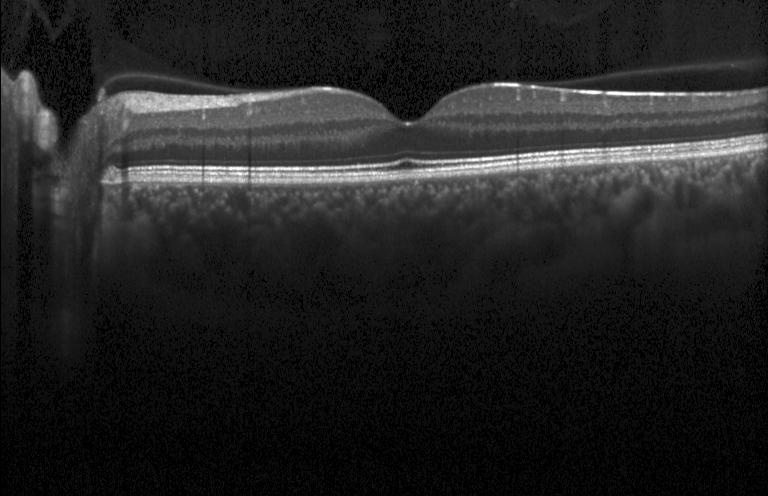 Optical coherence tomography B-scan. Assessment: no choroidal neovascularization, diabetic macular edema, or drusen.